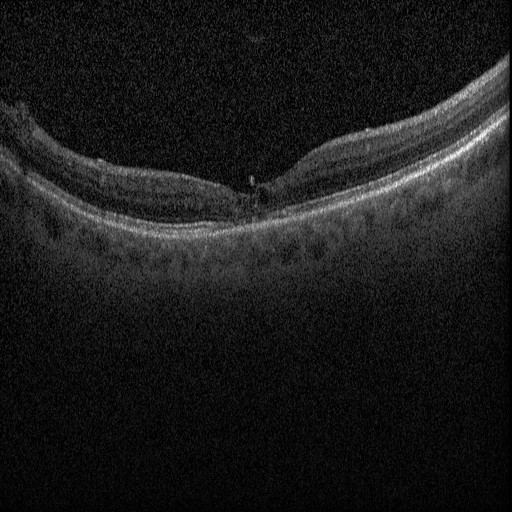

Macular scan. OCT B-scan. Spectral-domain OCT. Finding: DME.